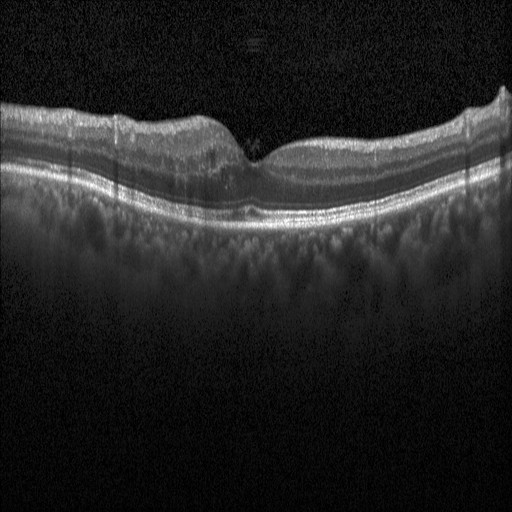
Instrument: Heidelberg Spectralis, OCT line scan.
Diagnosis: diabetic macular edema.